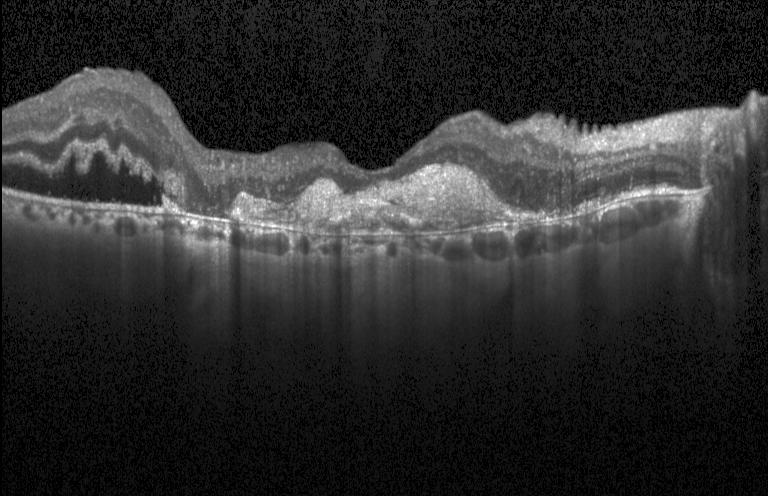

OCT scan showing a choroidal neovascular membrane.